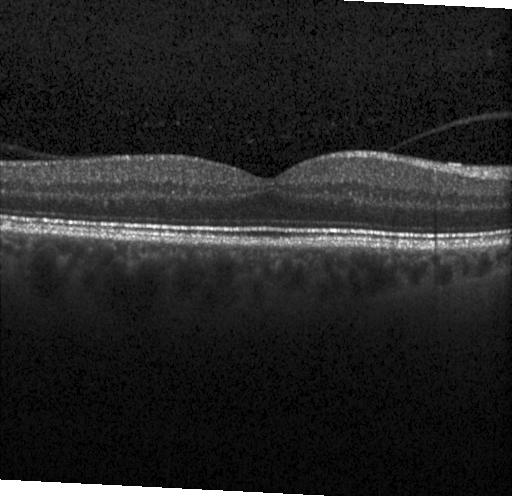

Through the macula · retinal OCT B-scan · Heidelberg Spectralis · spectral-domain optical coherence tomography
The scan shows no evidence of CNV, DME, or drusen.